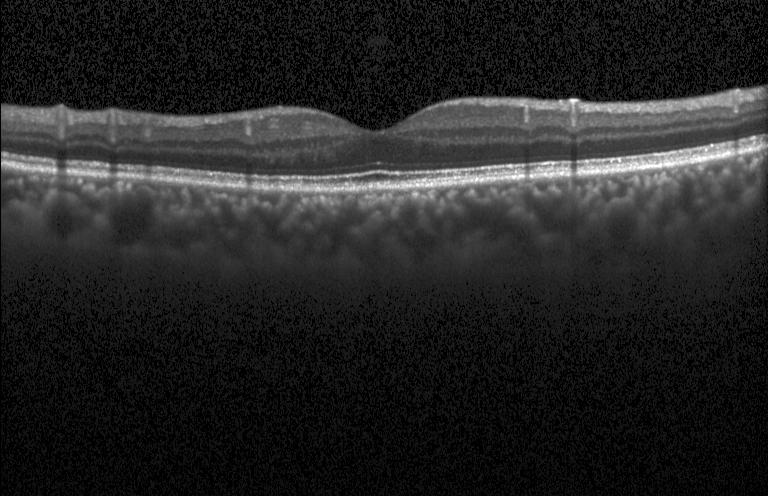

Macular OCT: no choroidal neovascularization, diabetic macular edema, or drusen.